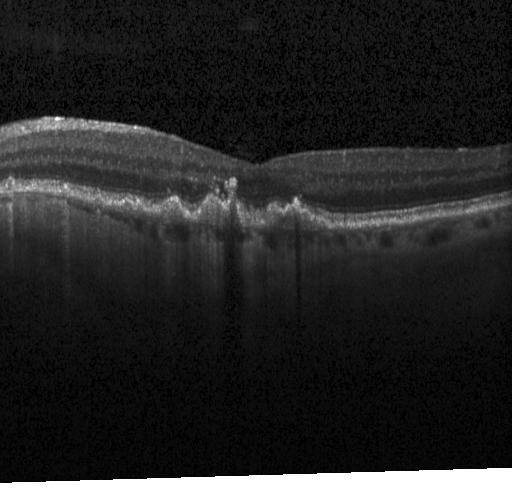
OCT B-scan showing drusen.